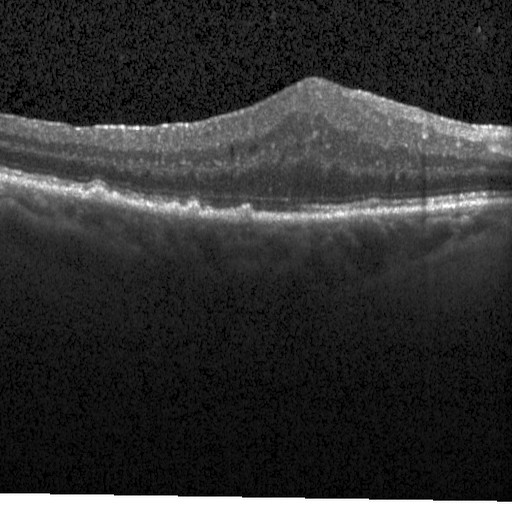 Diagnosis: diabetic macular edema.